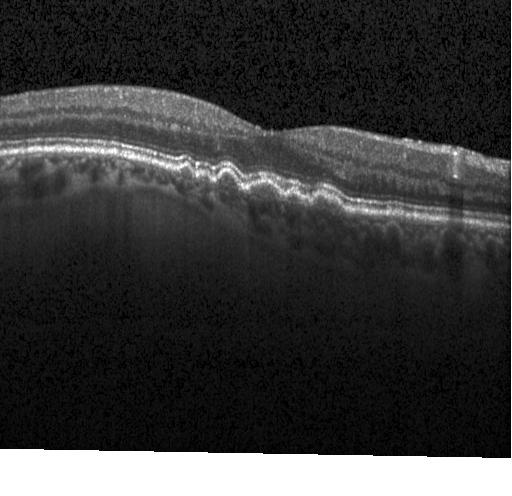

OCT line scan, Heidelberg Spectralis OCT system. Impression: multiple drusen.